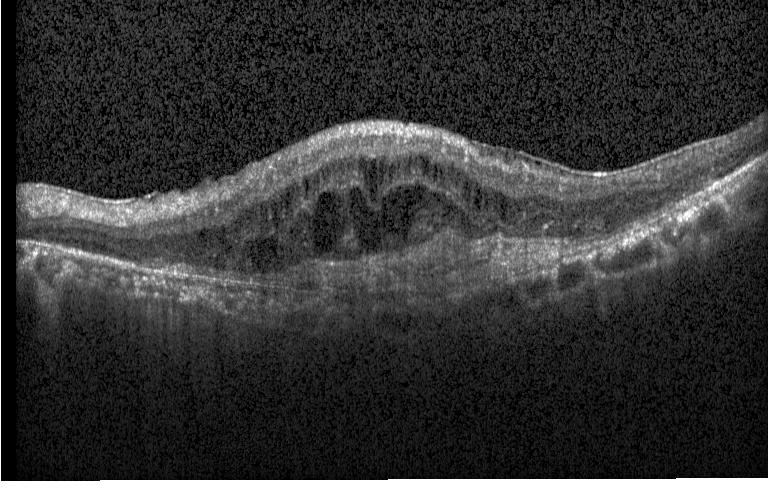 Diagnosis: choroidal neovascularization.